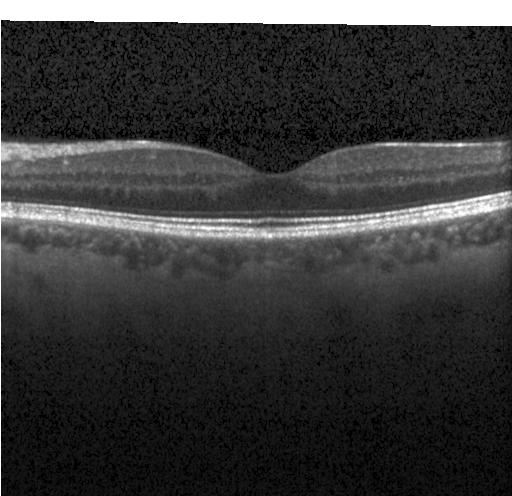
SD-OCT, optical coherence tomography scan — Impression: no choroidal neovascularization, no diabetic macular edema, and no drusen.